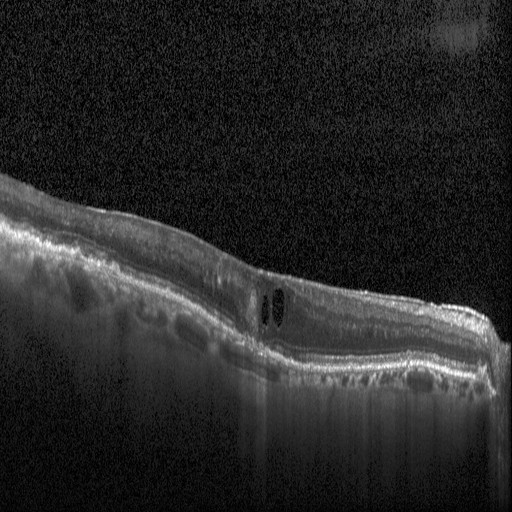 Retinal OCT cross-section · Heidelberg Spectralis · spectral-domain optical coherence tomography · horizontal scan through the fovea
Diagnosis: DME.